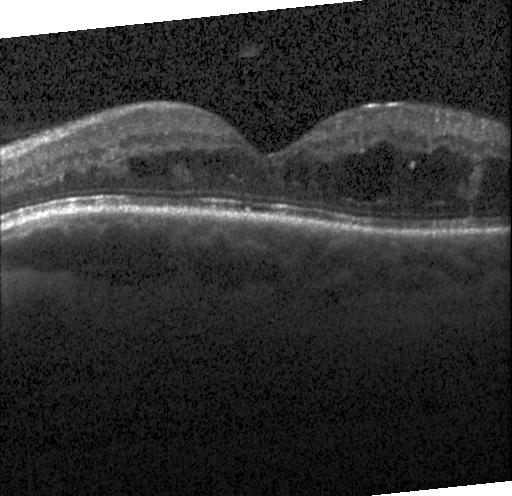
Diagnosis: diabetic macular edema (DME).